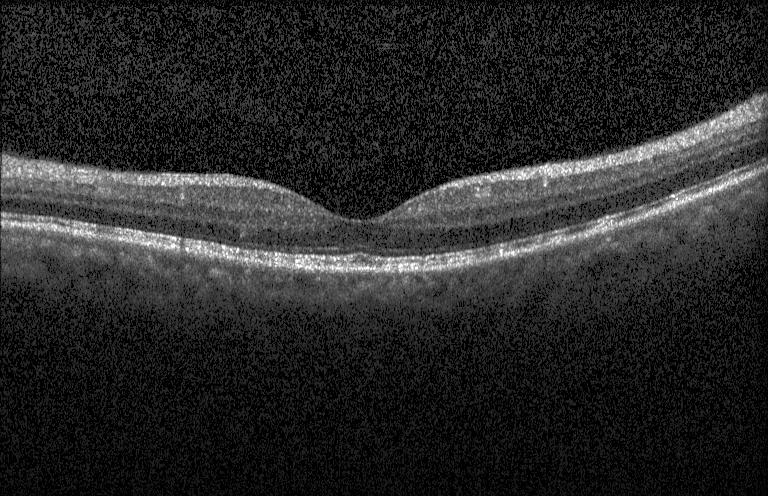
Heidelberg Spectralis, optical coherence tomography B-scan — Impression: no evidence of choroidal neovascularization, diabetic macular edema, or drusen.